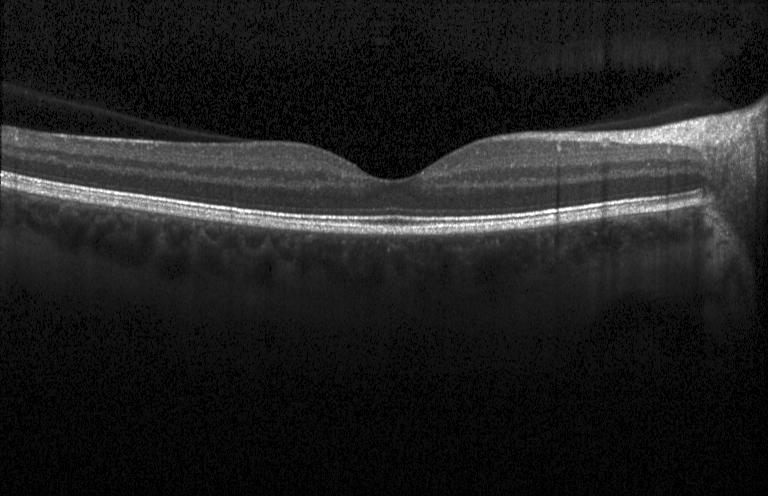
Optical coherence tomography B-scan. Acquired on a Heidelberg Spectralis
No evidence of CNV, DME, or drusen.